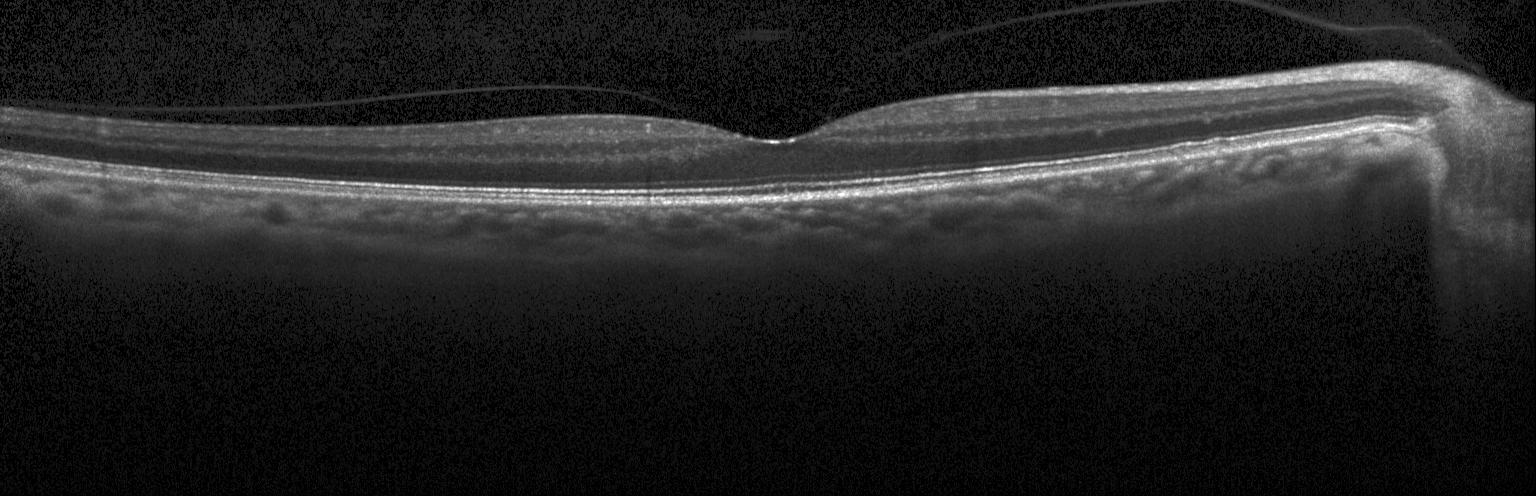 OCT line scan — Macular OCT: no evidence of choroidal neovascularization, diabetic macular edema, or drusen.